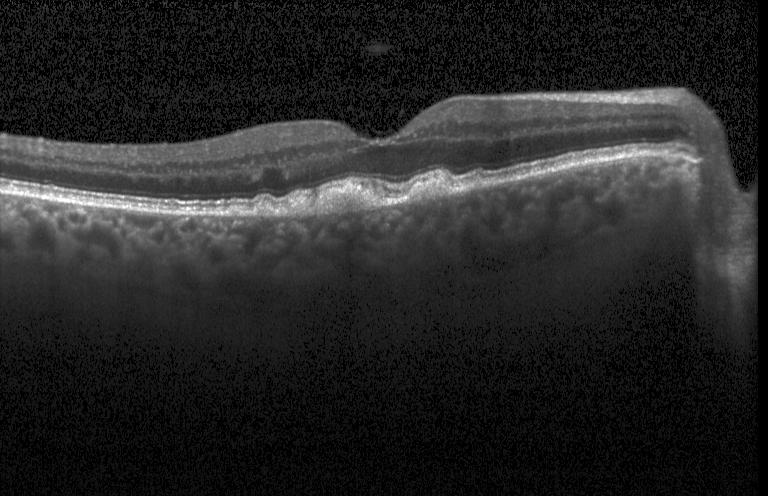
Heidelberg Spectralis, optical coherence tomography scan, centered on the fovea — Diagnosis: a choroidal neovascular membrane.